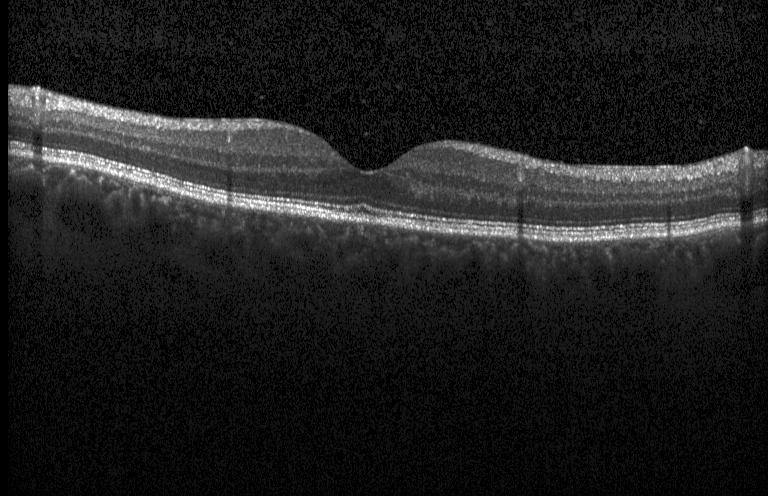
Heidelberg Spectralis OCT system, spectral-domain optical coherence tomography, macular scan, optical coherence tomography scan
Assessment: no evidence of CNV, DME, or drusen.